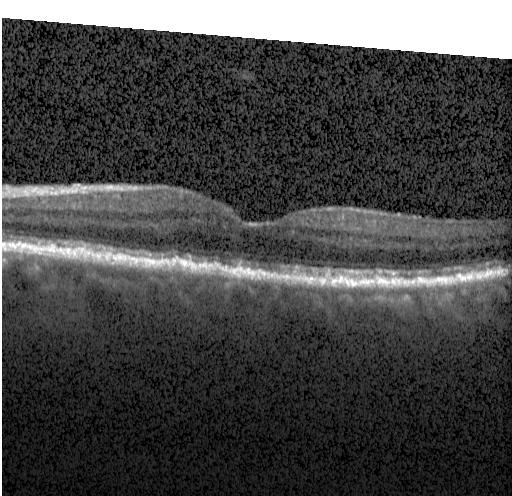
Optical coherence tomography scan. Heidelberg Spectralis. SD-OCT.
The scan shows multiple drusen.